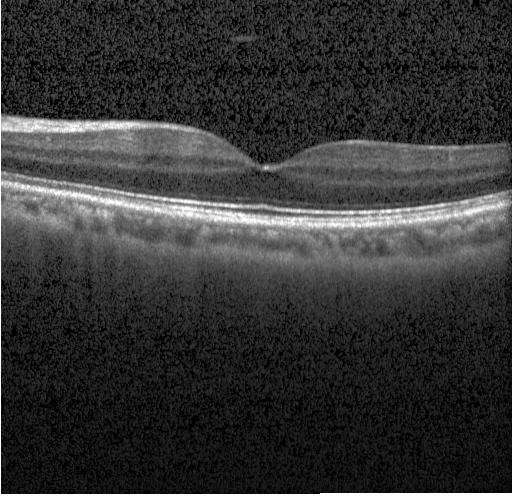
Acquired on a Heidelberg Spectralis; OCT line scan
Impression: no evidence of choroidal neovascularization, diabetic macular edema, or drusen.